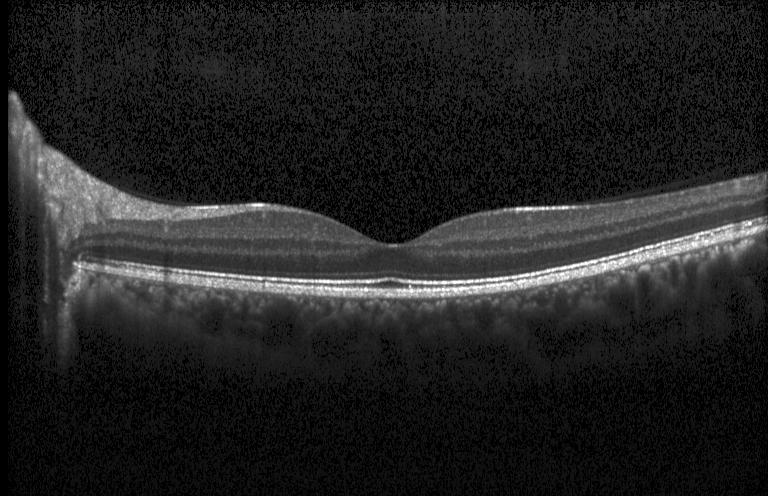
OCT B-scan — No choroidal neovascularization, diabetic macular edema, or drusen.